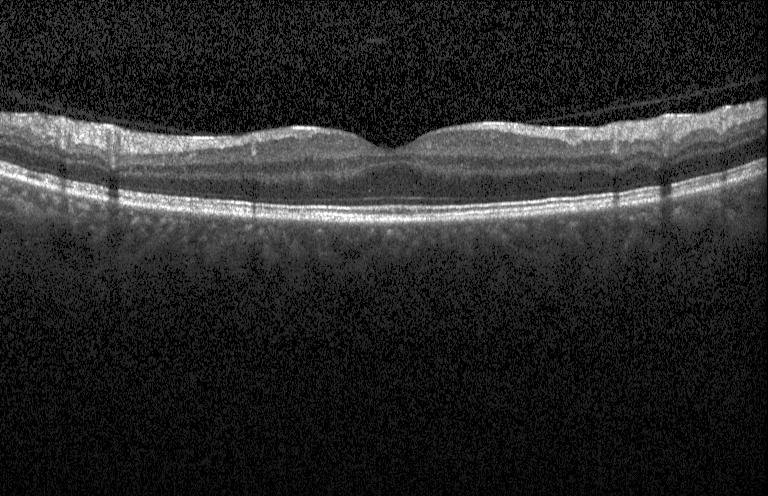
OCT B-scan — OCT finding: no evidence of choroidal neovascularization, diabetic macular edema, or drusen.